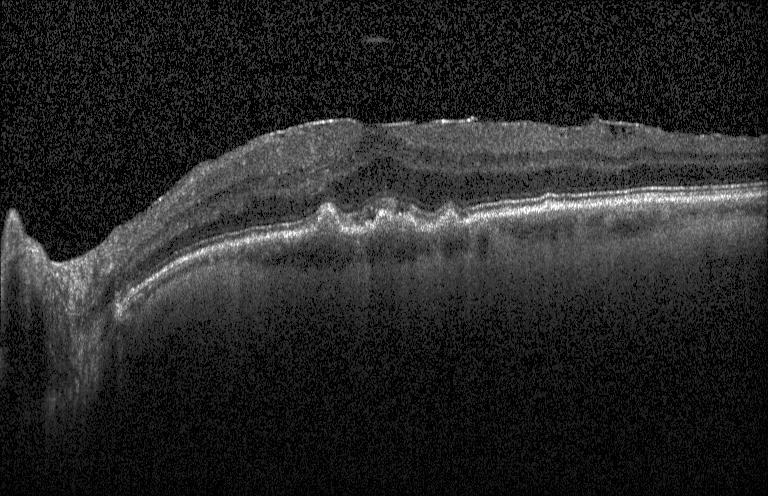

Drusen.